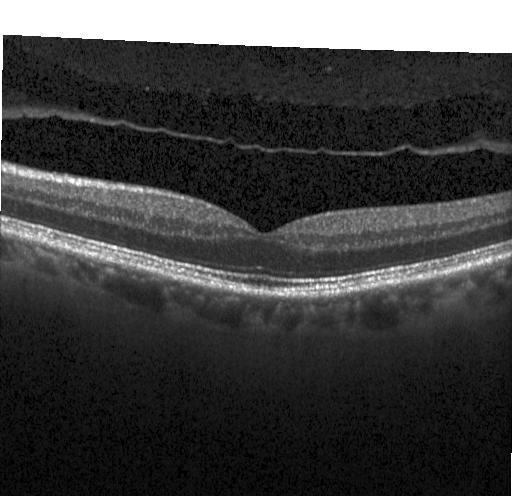 Fovea-centered · optical coherence tomography B-scan · Heidelberg Spectralis · SD-OCT
Finding: no CNV, DME, or drusen.